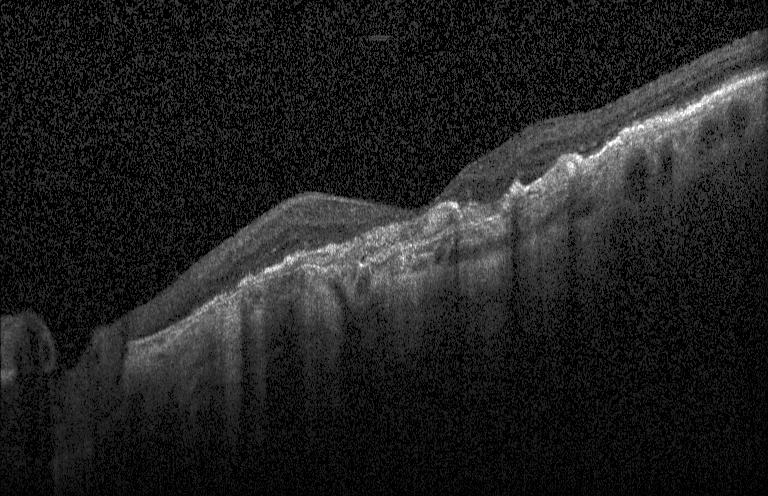
Horizontal scan through the fovea; optical coherence tomography scan; SD-OCT. Choroidal neovascularization (CNV).